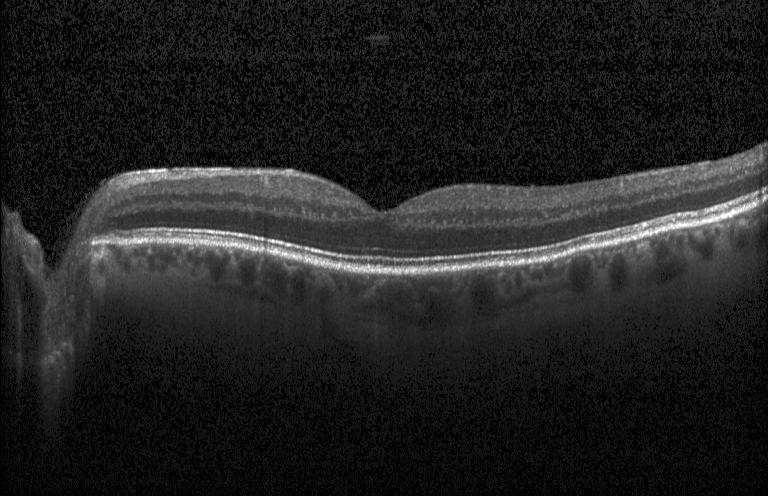 Assessment: no evidence of choroidal neovascularization, diabetic macular edema, or drusen.